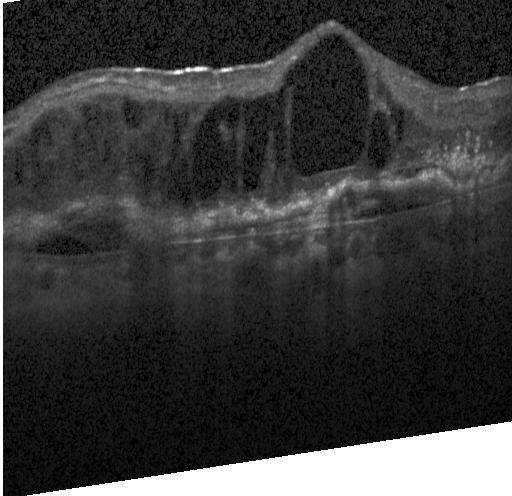
Through the macula · optical coherence tomography scan. The scan shows CNV.